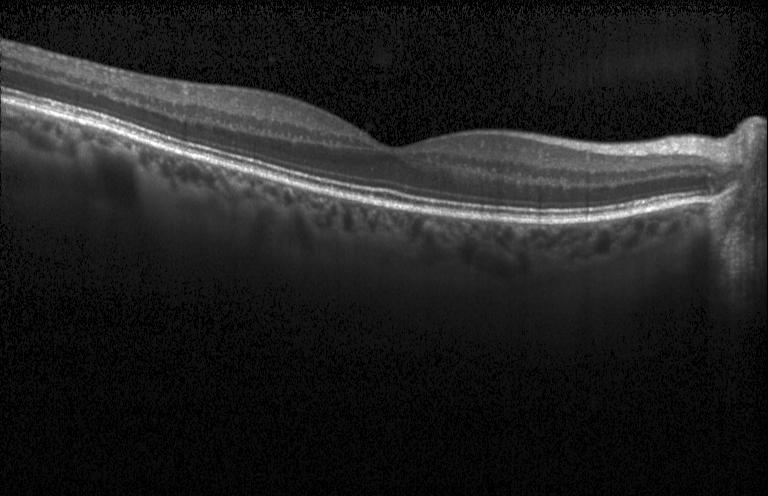

Retinal OCT B-scan
This B-scan demonstrates no choroidal neovascularization, diabetic macular edema, or drusen.